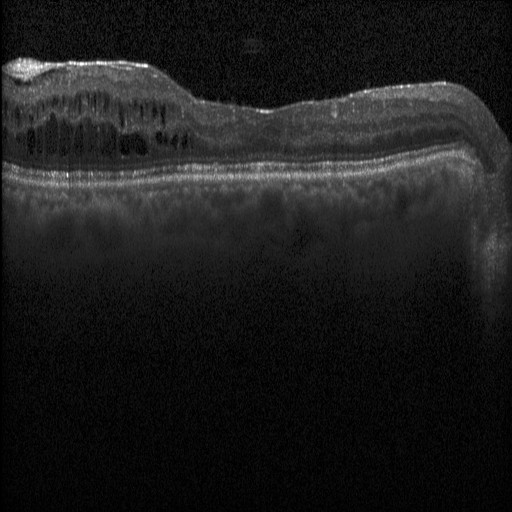 Impression: diabetic macular edema (DME).